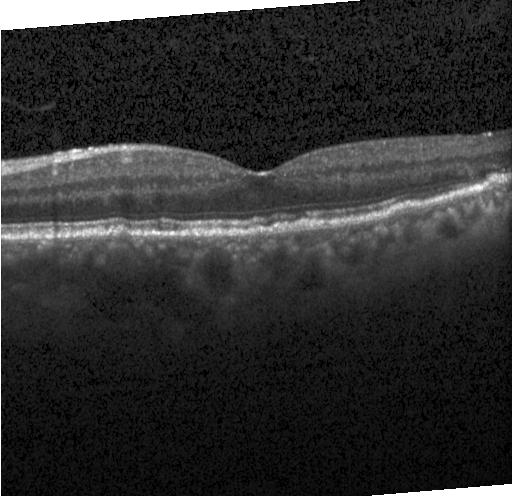 Spectral-domain optical coherence tomography. Macular scan. Retinal OCT cross-section. Drusen.